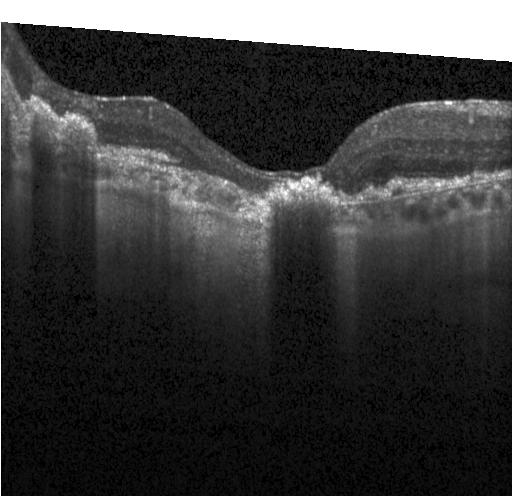

The scan shows choroidal neovascularization (CNV).